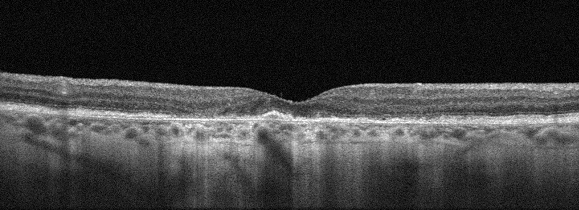
Optical coherence tomography scan · oculus sinister — Age-related macular degeneration.